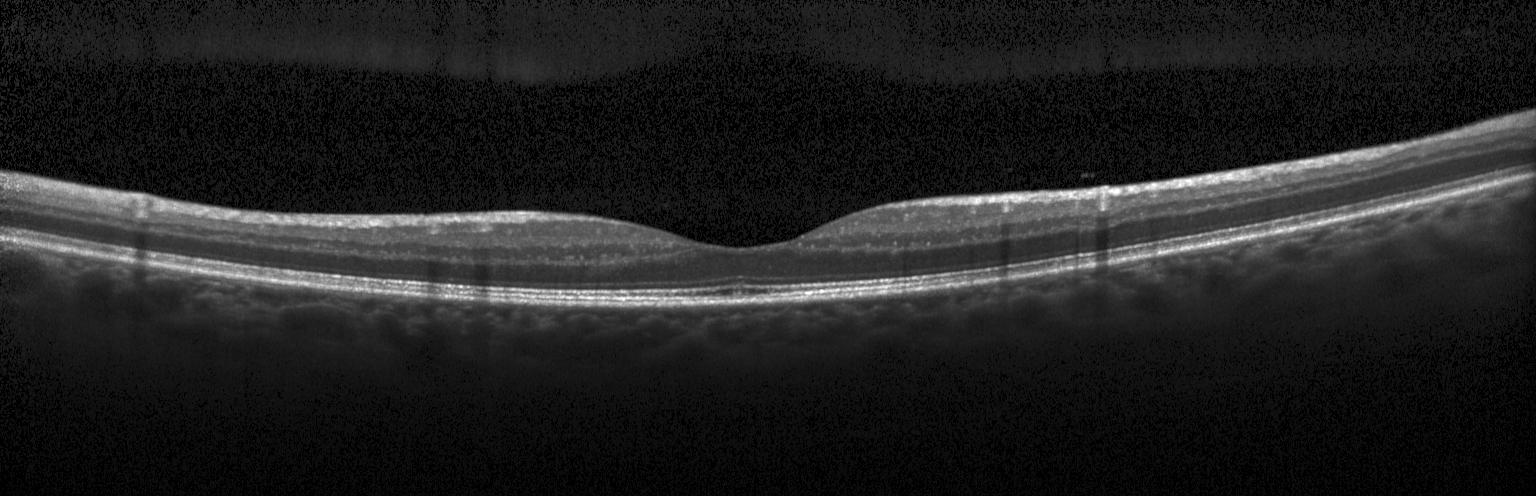

Spectral-domain OCT, centered on the fovea, acquired on a Heidelberg Spectralis, retinal OCT B-scan. Dx: neither choroidal neovascularization, diabetic macular edema, nor drusen.